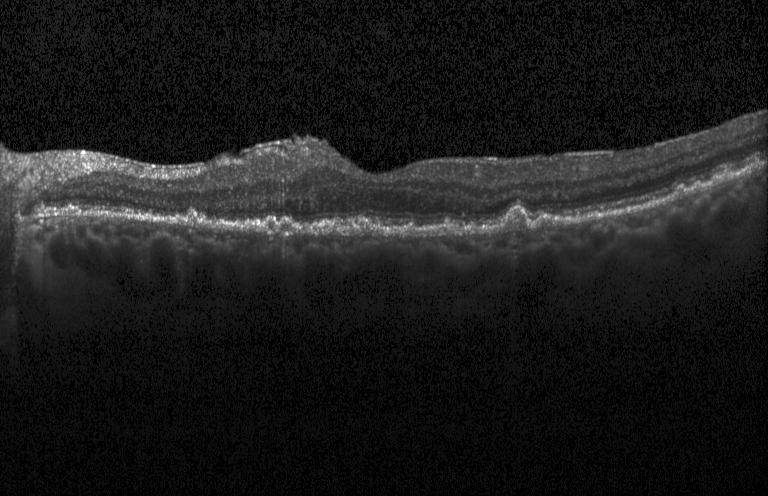 Spectral-domain OCT B-scan: multiple drusen.